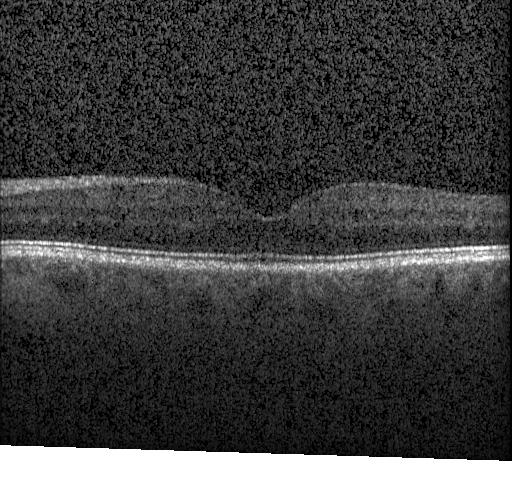 Retinal OCT cross-section · Heidelberg Spectralis. Impression: neither choroidal neovascularization, diabetic macular edema, nor drusen.